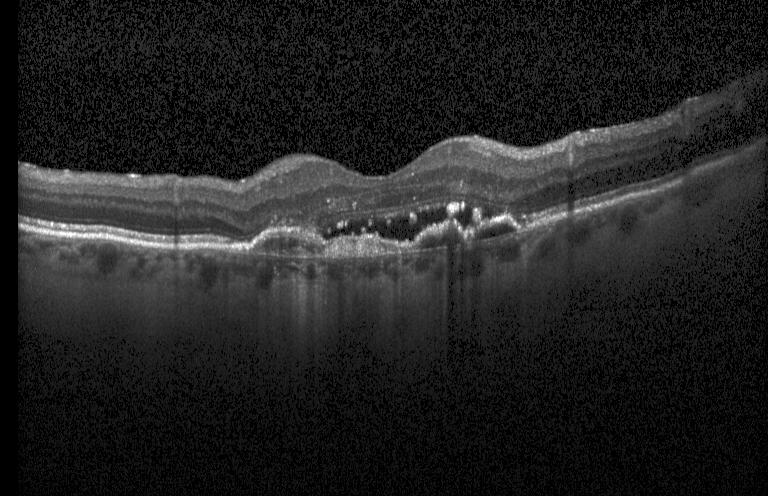
Diagnosis: a choroidal neovascular membrane.